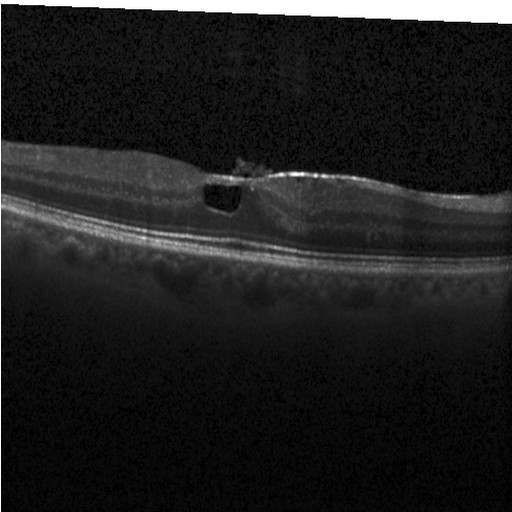

Retinal OCT cross-section showing diabetic macular edema (DME).